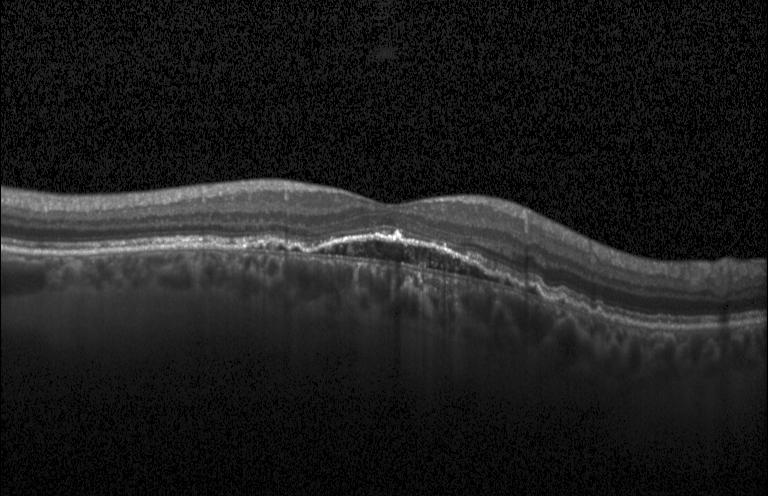
Spectral-domain OCT B-scan: a choroidal neovascular membrane.